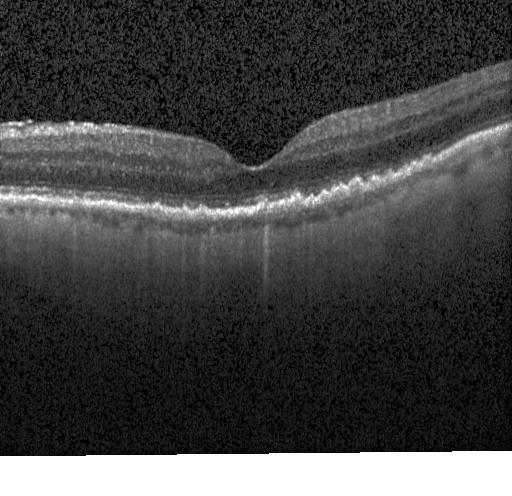 Retinal OCT cross-section; through the macula; SD-OCT
Impression: drusen.